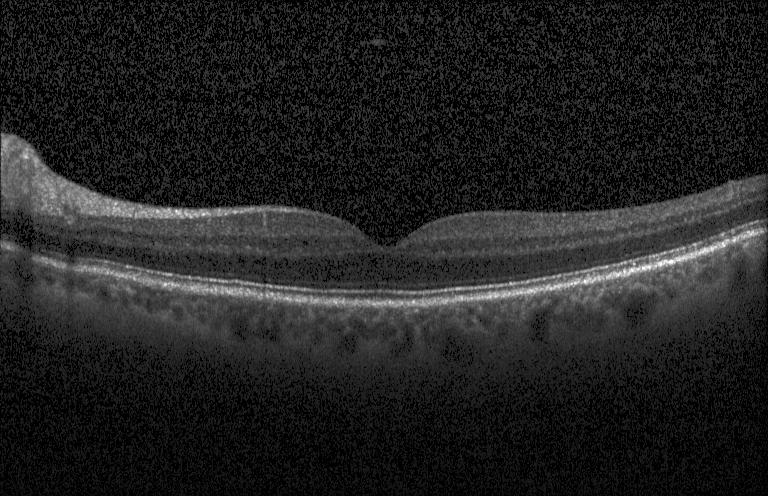

Spectral-domain OCT, retinal OCT cross-section, Heidelberg Spectralis OCT system, fovea-centered
Macular OCT: no choroidal neovascularization, diabetic macular edema, or drusen.